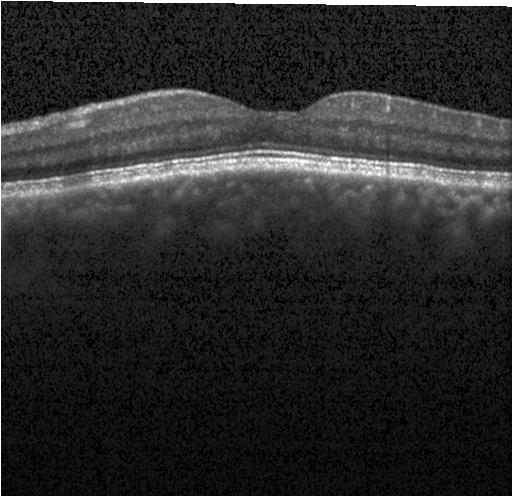 The scan shows neither CNV, DME, nor drusen.